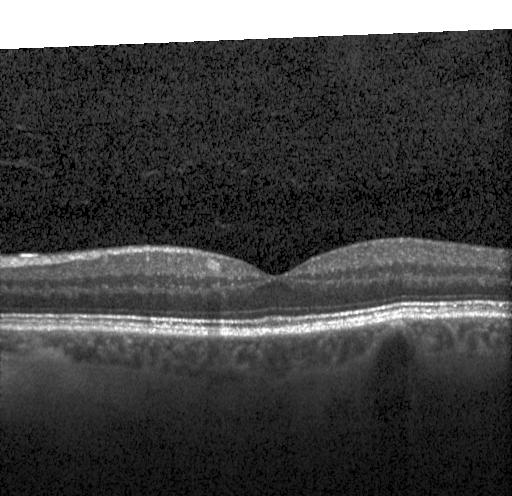

OCT line scan
Finding: no CNV, DME, or drusen.